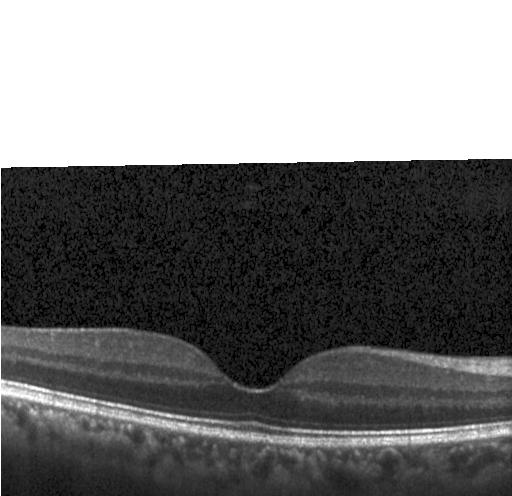
Impression: no choroidal neovascularization, no diabetic macular edema, and no drusen.